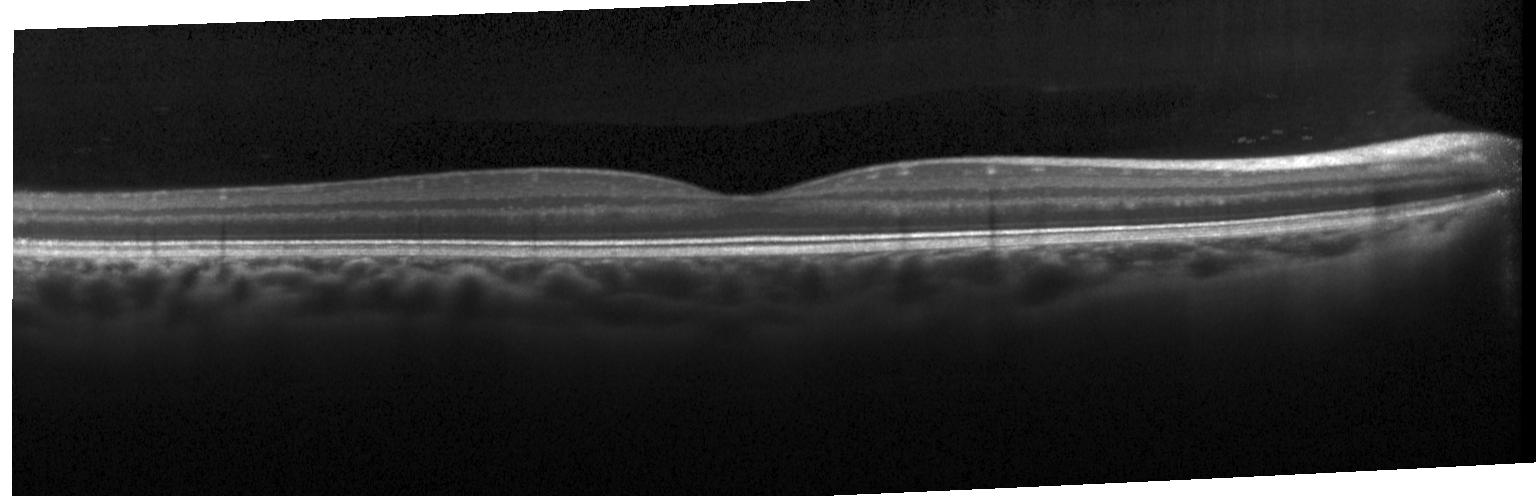
OCT B-scan.
Finding: no choroidal neovascularization, diabetic macular edema, or drusen.